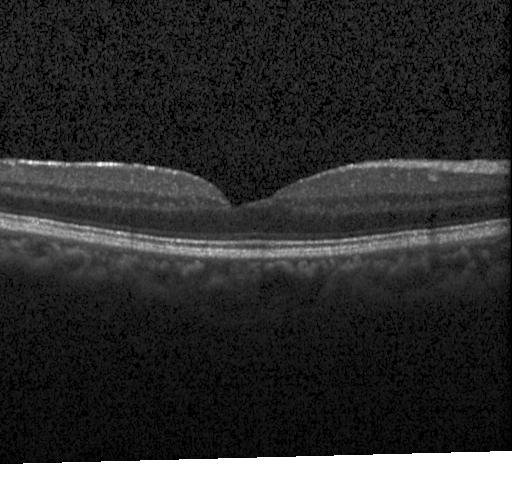
Centered on the fovea; optical coherence tomography scan — Diagnosis: no choroidal neovascularization, diabetic macular edema, or drusen.